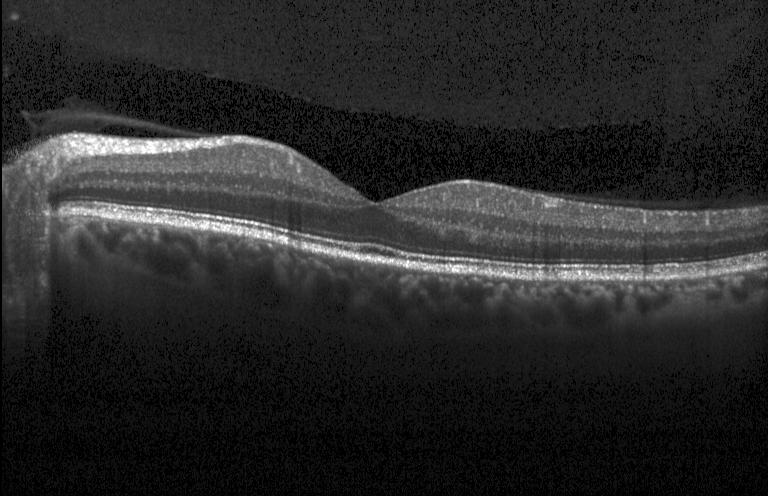 Impression: neither choroidal neovascularization, diabetic macular edema, nor drusen.